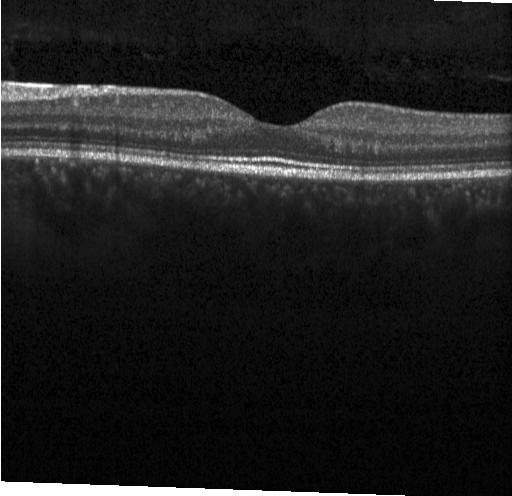 Retinal OCT B-scan — No evidence of choroidal neovascularization, diabetic macular edema, or drusen.